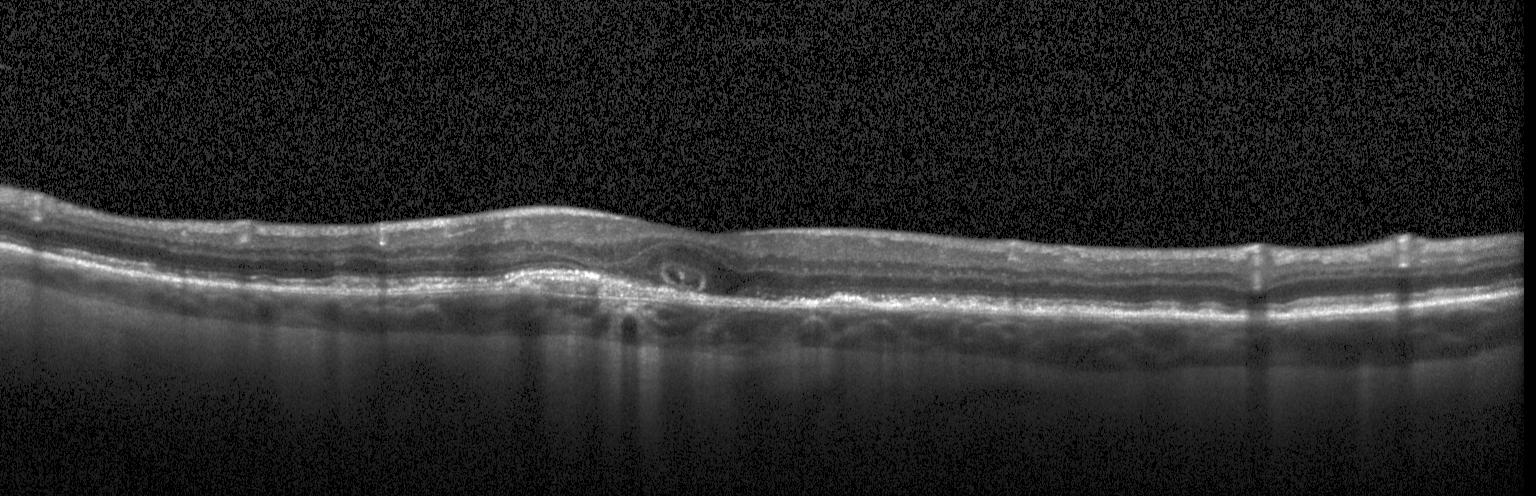

Horizontal scan through the fovea; spectral-domain OCT; optical coherence tomography scan — Finding: choroidal neovascularization (CNV).